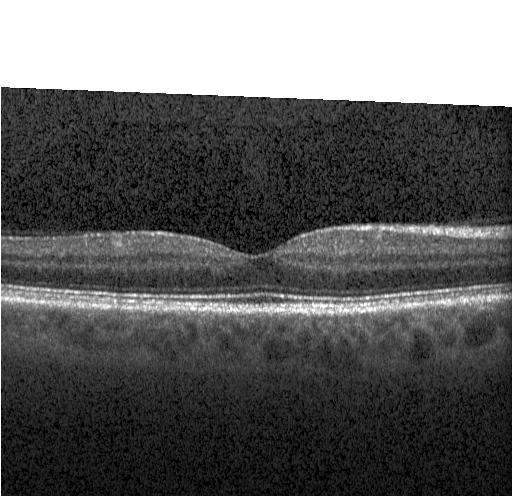

SD-OCT, OCT B-scan, acquired on a Heidelberg Spectralis, macular scan. Impression: neither choroidal neovascularization, diabetic macular edema, nor drusen.